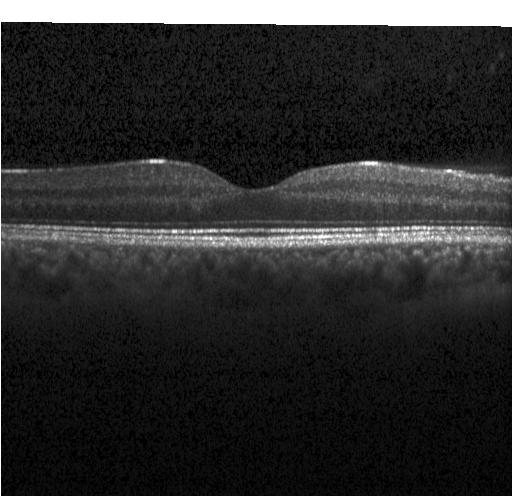
Retinal OCT cross-section.
Diagnosis: no choroidal neovascularization, no diabetic macular edema, and no drusen.